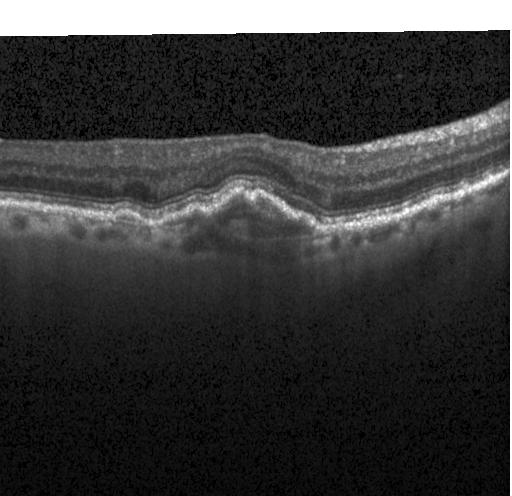
Finding: CNV.